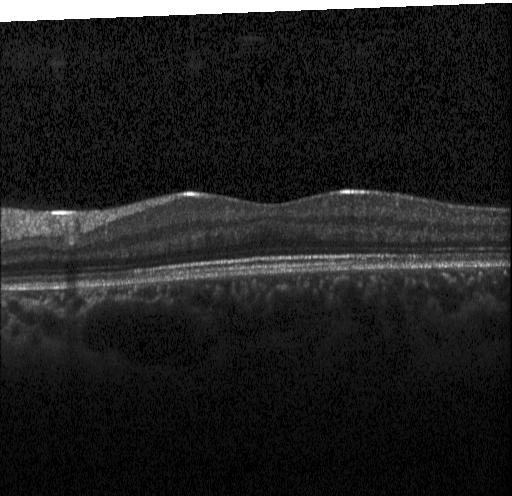

Macular OCT: no evidence of CNV, DME, or drusen.